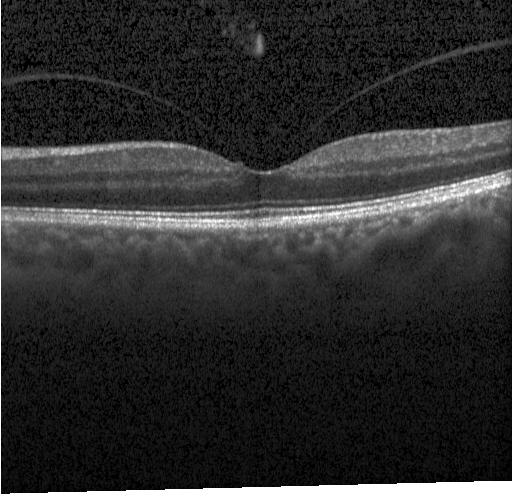

SD-OCT · acquired on a Heidelberg Spectralis · OCT line scan. Macular OCT: no CNV, no DME, and no drusen.